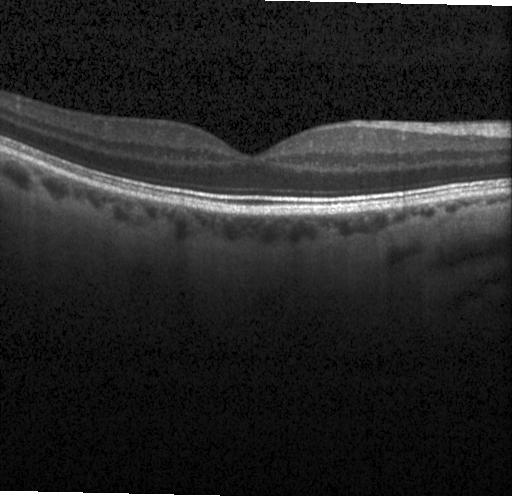
Retinal OCT cross-section showing no evidence of choroidal neovascularization, diabetic macular edema, or drusen.